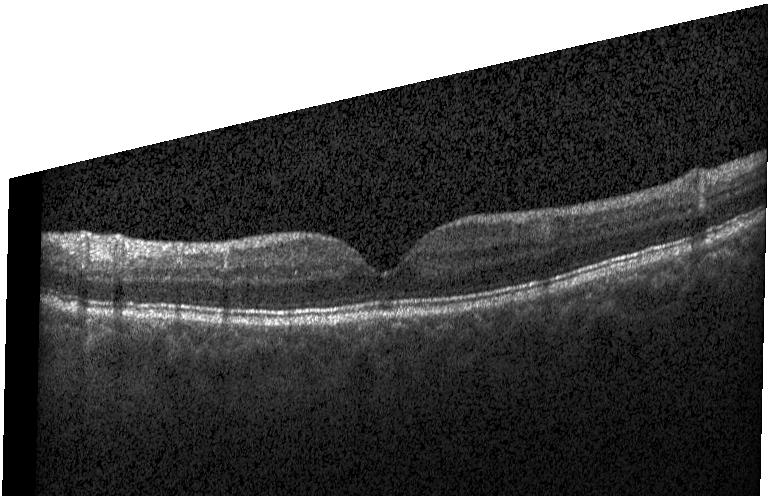 Heidelberg Spectralis, retinal OCT B-scan, macular scan, SD-OCT.
Impression: no evidence of choroidal neovascularization, diabetic macular edema, or drusen.